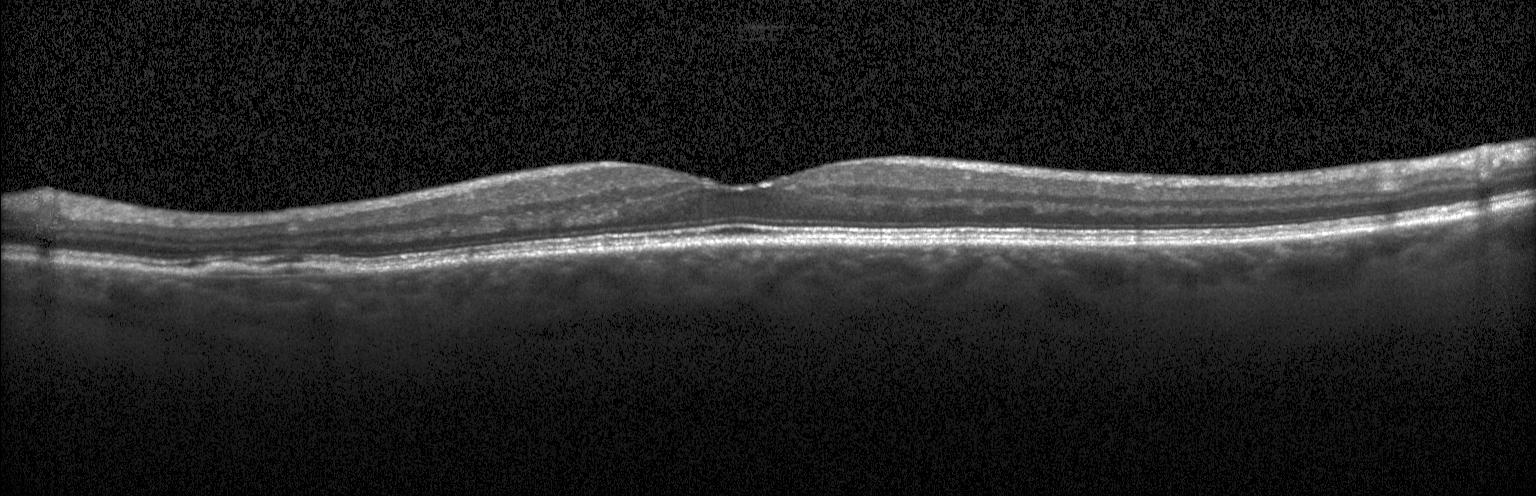 Retinal OCT cross-section
The scan shows choroidal neovascularization (CNV).